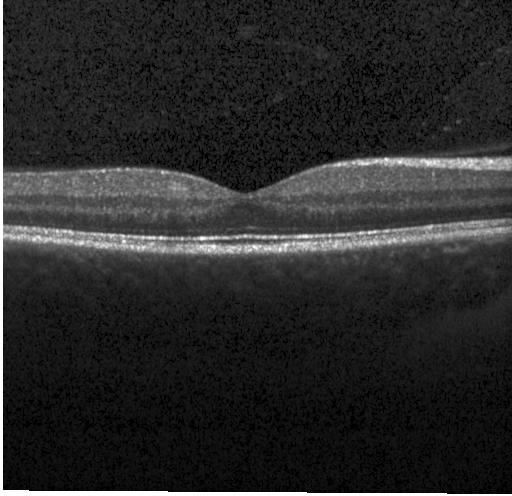 Retinal OCT cross-section; spectral-domain OCT
Finding: neither choroidal neovascularization, diabetic macular edema, nor drusen.